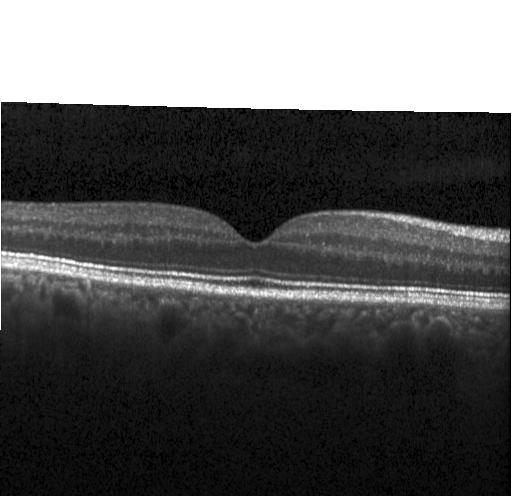 Optical coherence tomography B-scan; fovea-centered; spectral-domain optical coherence tomography — Assessment: neither choroidal neovascularization, diabetic macular edema, nor drusen.